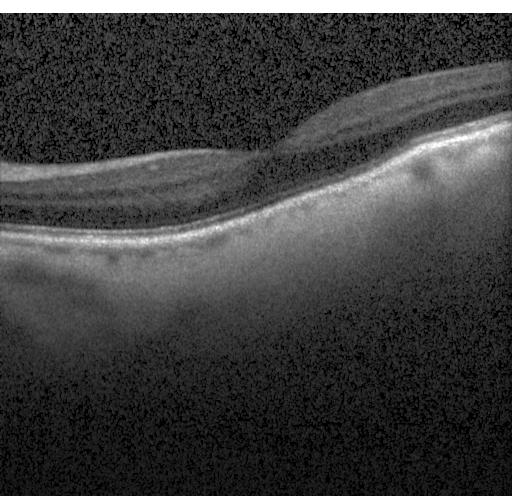 Instrument: Heidelberg Spectralis · centered on the fovea · optical coherence tomography B-scan · spectral-domain OCT. OCT finding: no choroidal neovascularization, no diabetic macular edema, and no drusen.